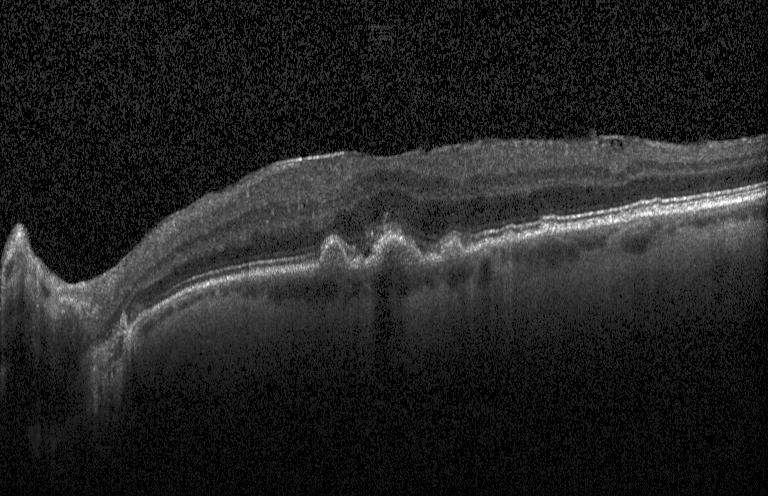

OCT scan showing multiple drusen.